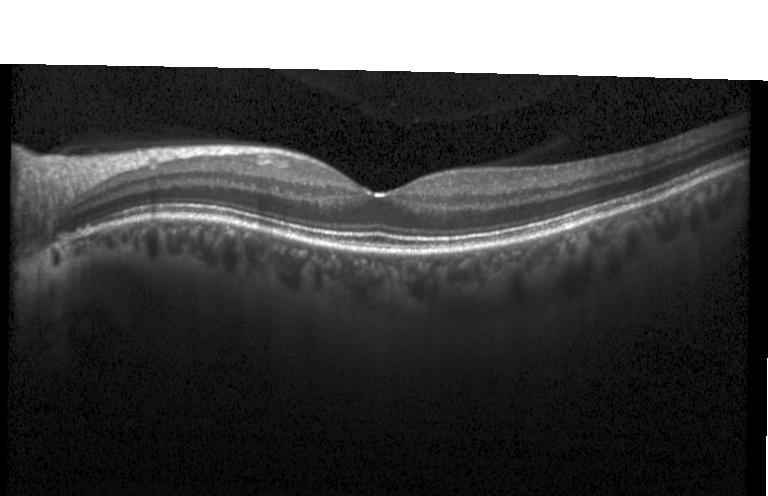
Optical coherence tomography B-scan · SD-OCT. The scan shows no choroidal neovascularization, diabetic macular edema, or drusen.